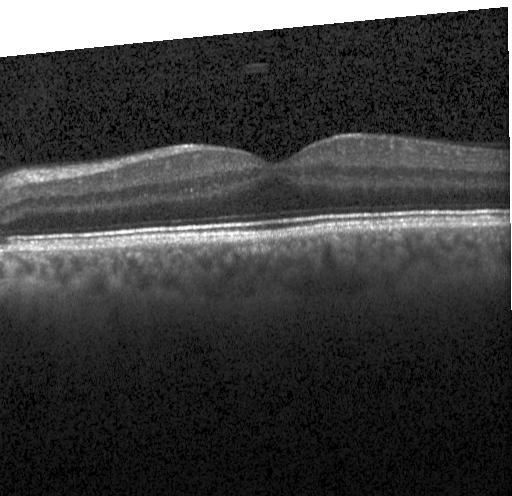 OCT B-scan. Acquired on a Heidelberg Spectralis. Impression: no choroidal neovascularization, no diabetic macular edema, and no drusen.